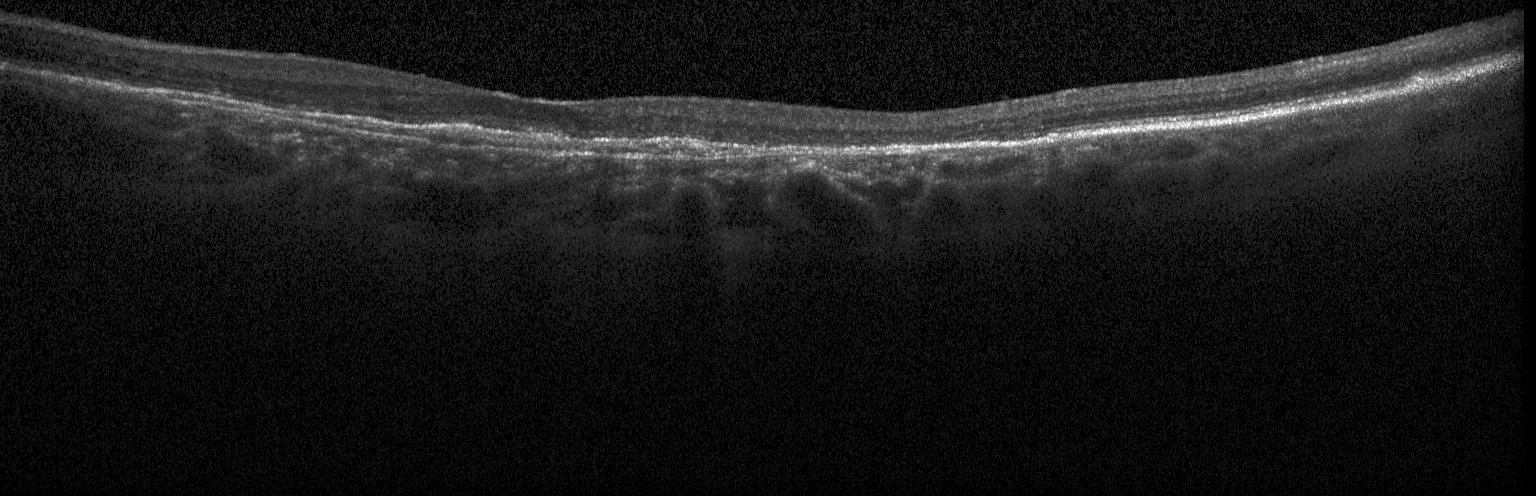 Acquired on a Heidelberg Spectralis; retinal OCT B-scan
Assessment: choroidal neovascularization (CNV).